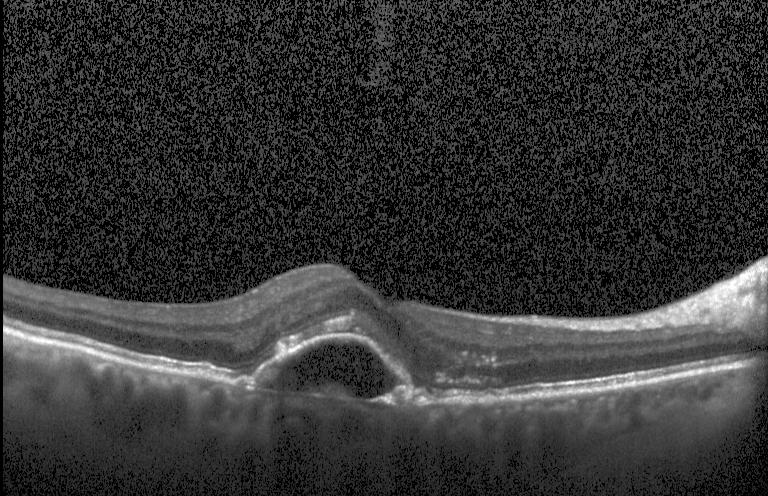 Finding: choroidal neovascularization.